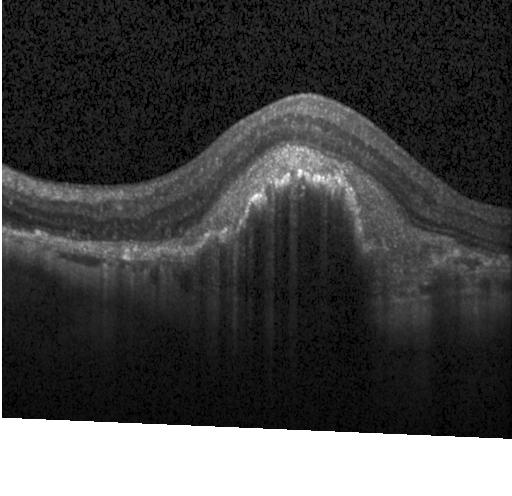 Finding: a choroidal neovascular membrane.